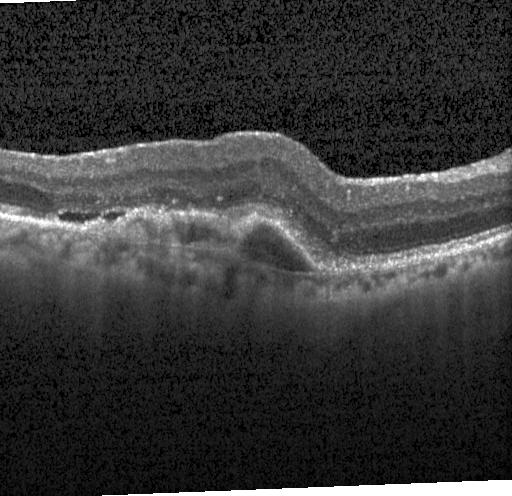
Spectral-domain optical coherence tomography; fovea-centered; acquired on a Heidelberg Spectralis; retinal OCT B-scan.
Impression: CNV.